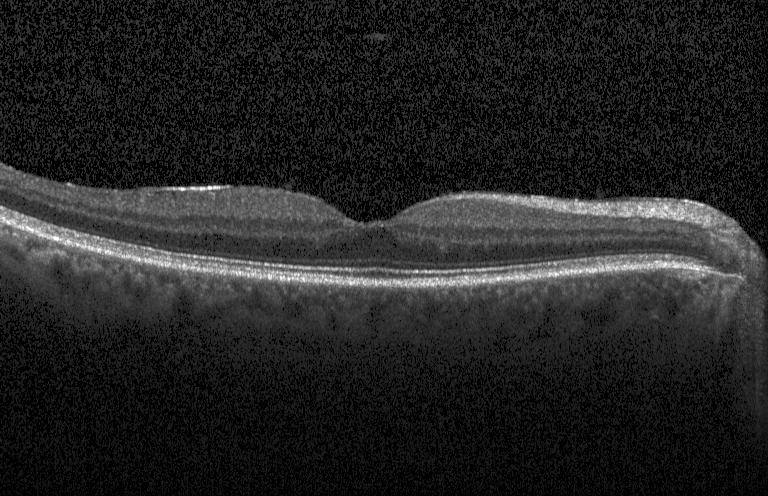 Diagnosis: no evidence of choroidal neovascularization, diabetic macular edema, or drusen.